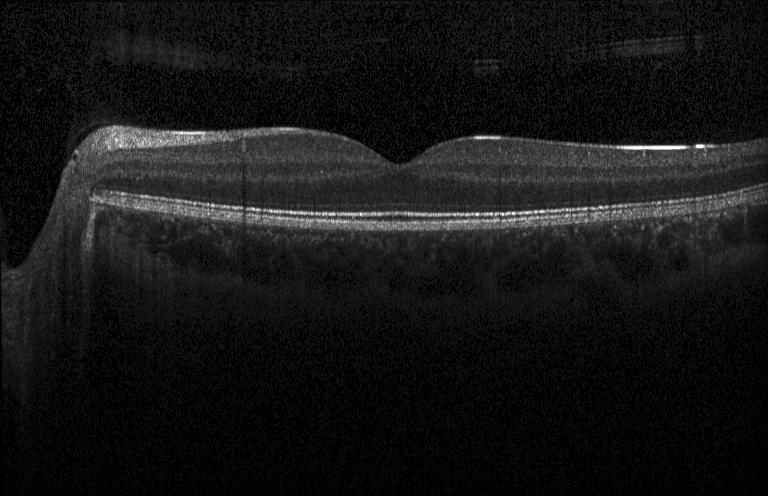

Retinal OCT B-scan. Fovea-centered. Spectral-domain OCT.
OCT finding: no evidence of choroidal neovascularization, diabetic macular edema, or drusen.